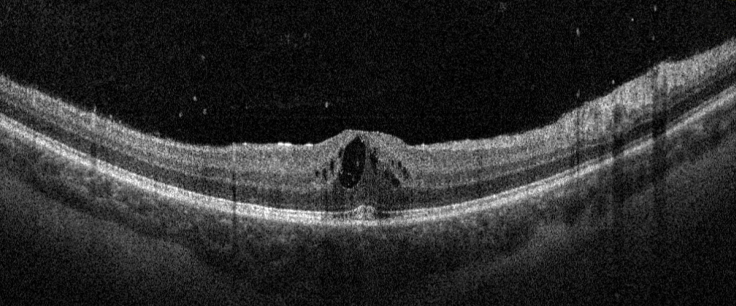 Impression: DME.